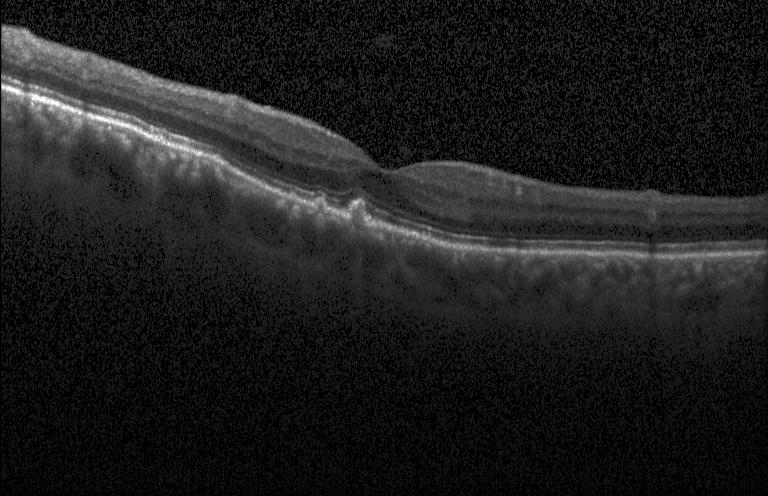 Impression: drusen.